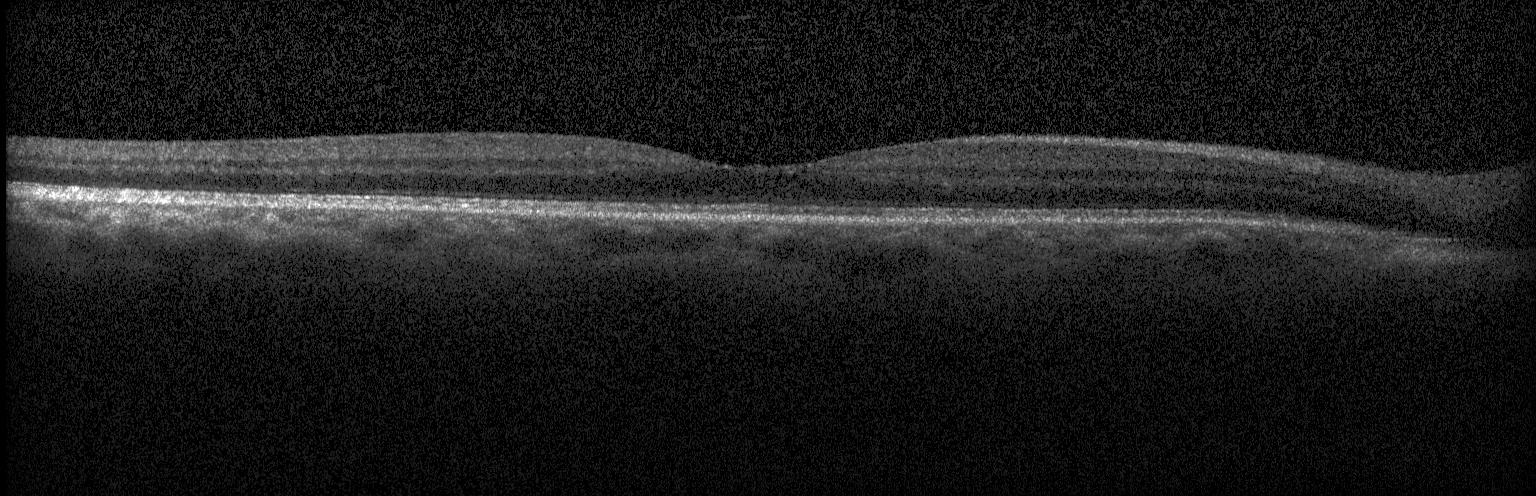
Macular OCT: neither choroidal neovascularization, diabetic macular edema, nor drusen.